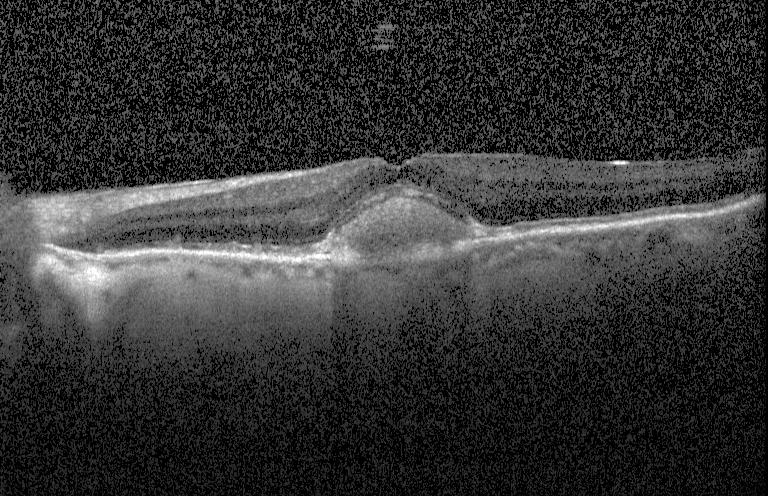 OCT B-scan. Through the macula.
Impression: a choroidal neovascular membrane.